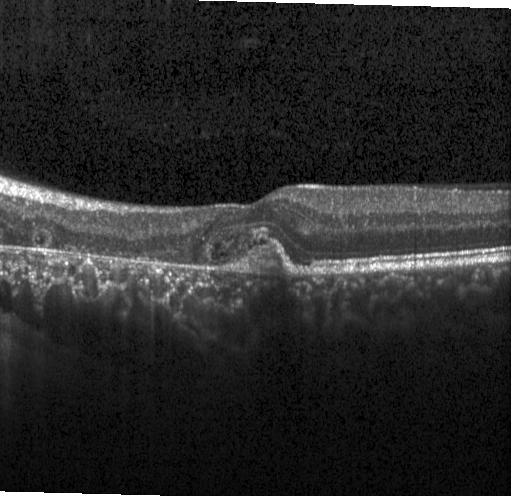 Spectral-domain optical coherence tomography, OCT B-scan, through the macula, Heidelberg Spectralis.
Macular OCT: CNV.